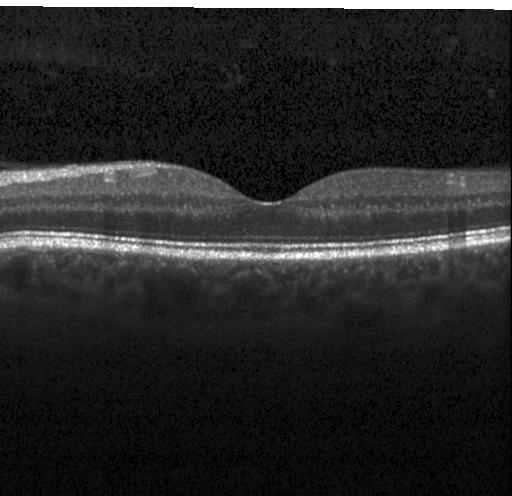 Optical coherence tomography B-scan, SD-OCT, Heidelberg Spectralis, through the macula.
Diagnosis: no evidence of choroidal neovascularization, diabetic macular edema, or drusen.